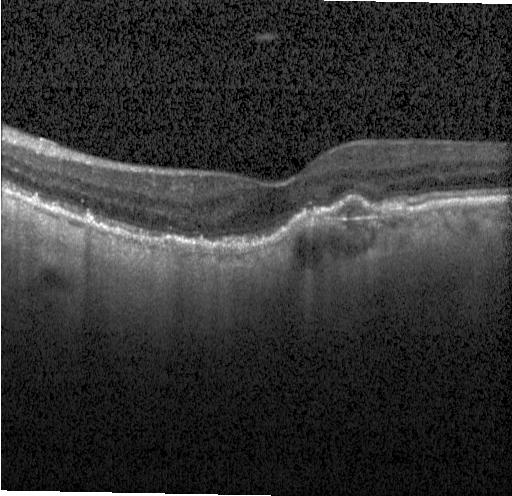

Retinal OCT cross-section — Impression: choroidal neovascularization (CNV).